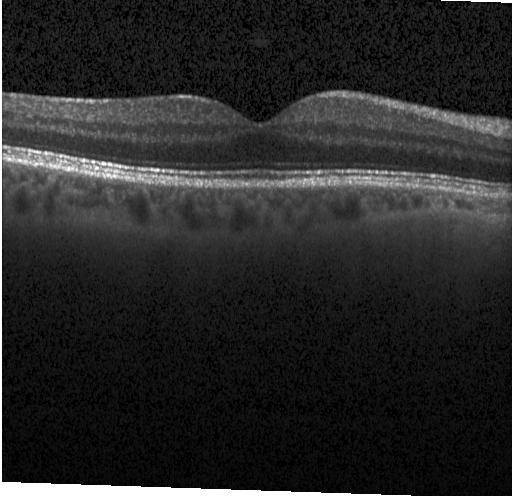
Retinal OCT B-scan. Diagnosis: no evidence of choroidal neovascularization, diabetic macular edema, or drusen.